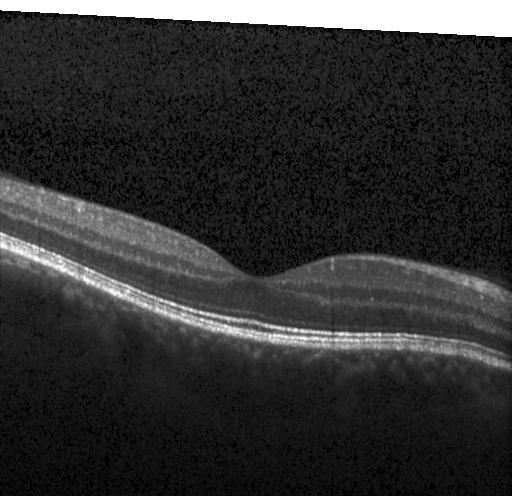
Retinal OCT cross-section; macular scan; SD-OCT
OCT finding: no choroidal neovascularization, no diabetic macular edema, and no drusen.